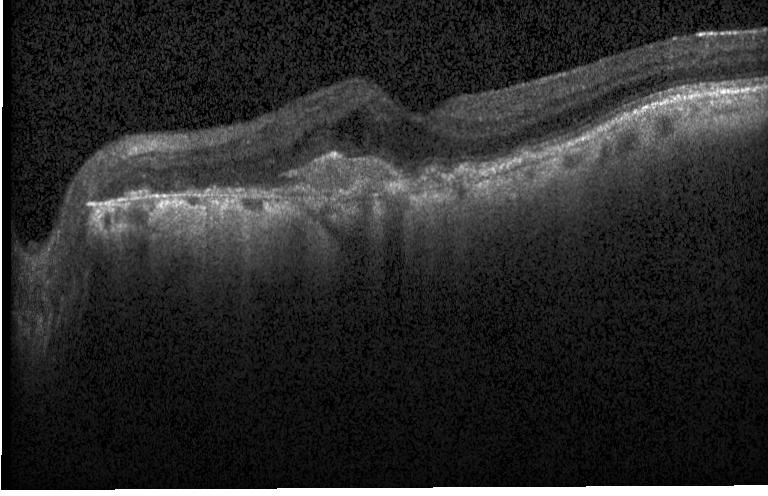

Macular scan. Acquired on a Heidelberg Spectralis. Optical coherence tomography B-scan. Spectral-domain optical coherence tomography
Finding: choroidal neovascularization (CNV).